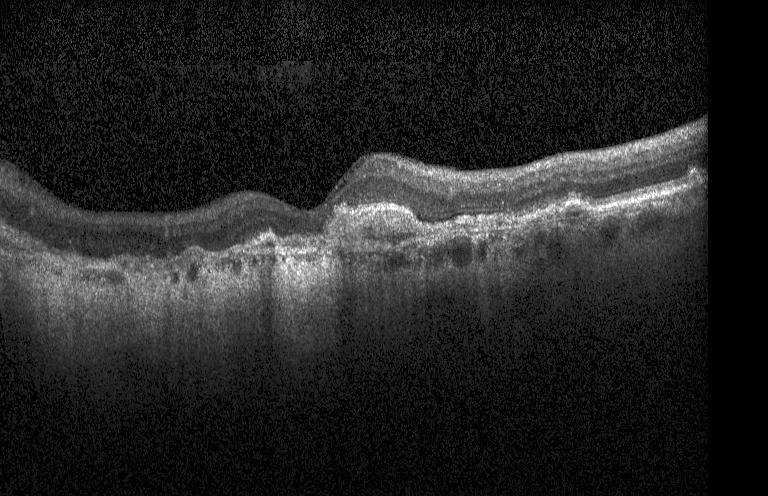 Through the macula, spectral-domain optical coherence tomography, optical coherence tomography scan.
Impression: a choroidal neovascular membrane.